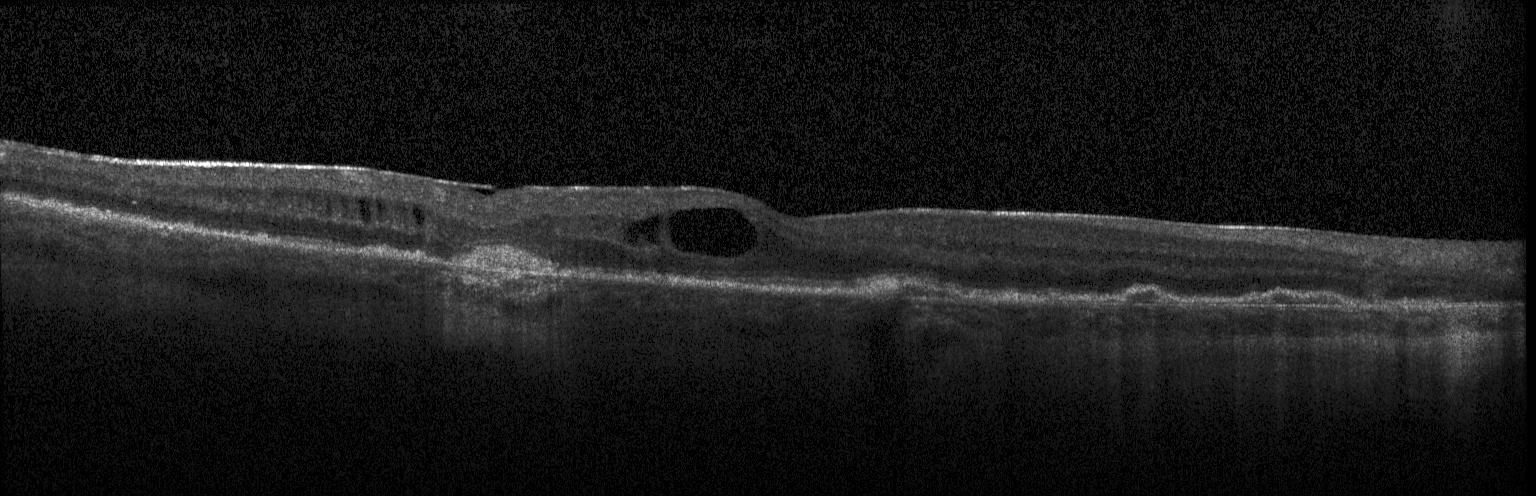

Finding: choroidal neovascularization (CNV).